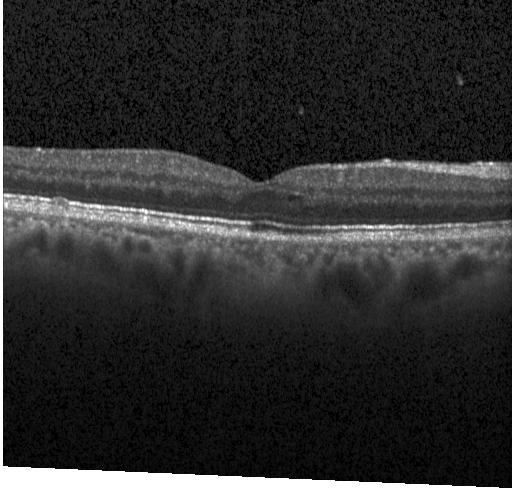 Retinal OCT B-scan; acquired on a Heidelberg Spectralis — Finding: no choroidal neovascularization, no diabetic macular edema, and no drusen.